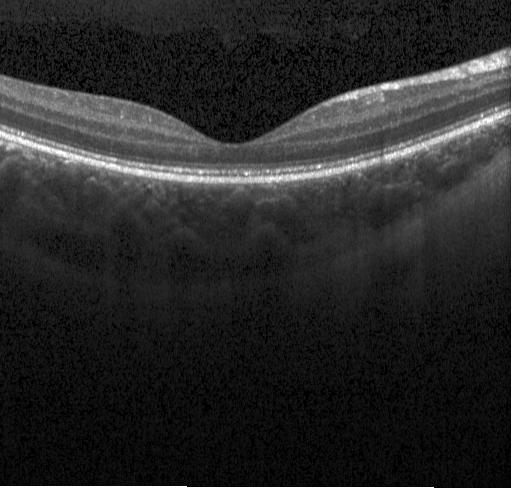 Heidelberg Spectralis; spectral-domain optical coherence tomography; optical coherence tomography scan. Finding: no choroidal neovascularization, no diabetic macular edema, and no drusen.